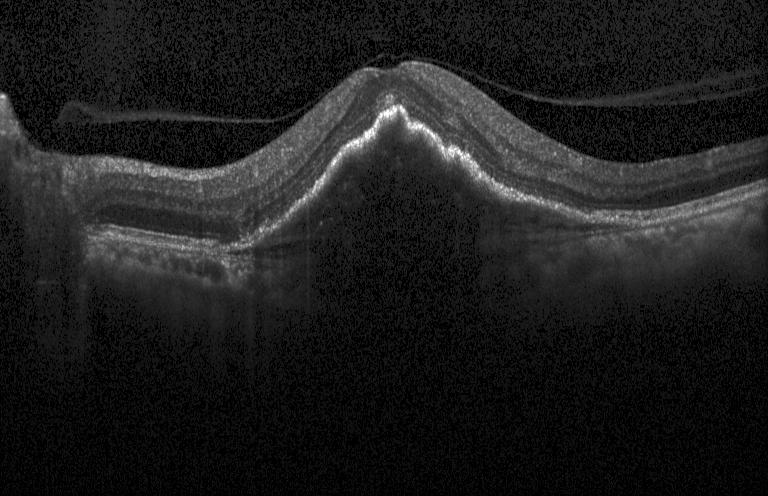

Finding: a choroidal neovascular membrane.